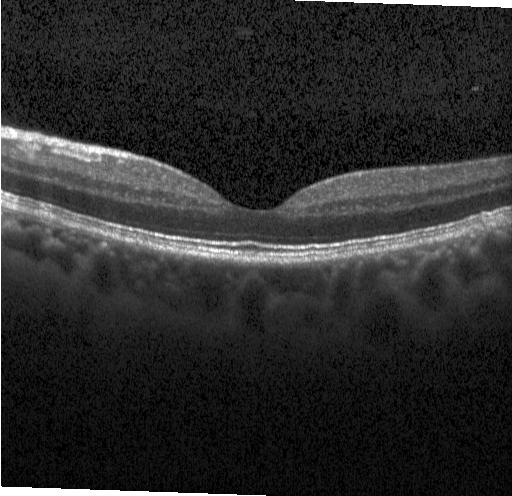

SD-OCT. Optical coherence tomography scan — Dx: no choroidal neovascularization, diabetic macular edema, or drusen.